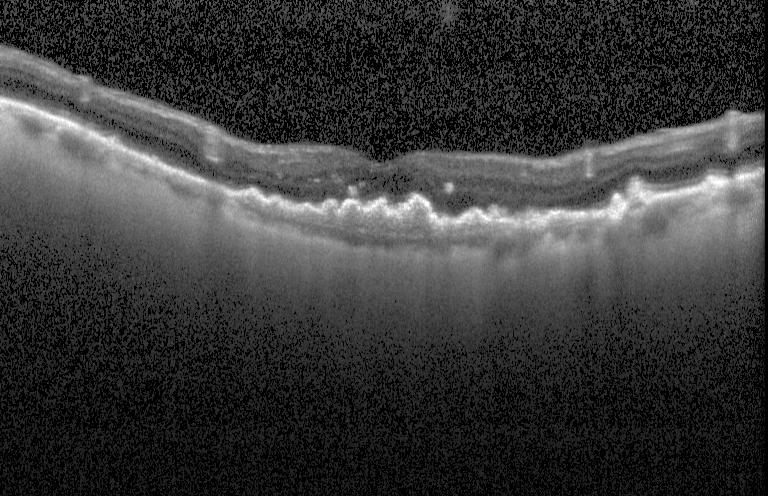 Diagnosis: CNV.